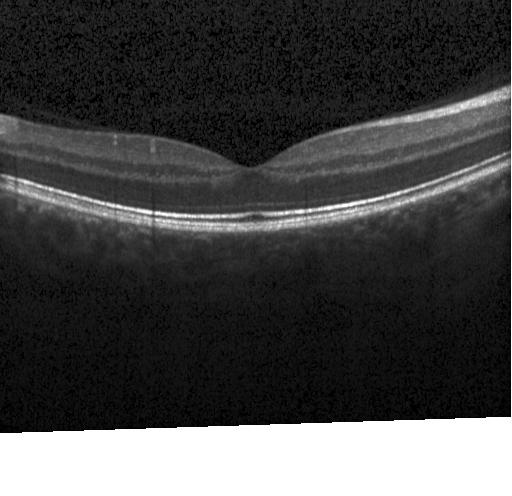
This B-scan demonstrates no evidence of CNV, DME, or drusen.